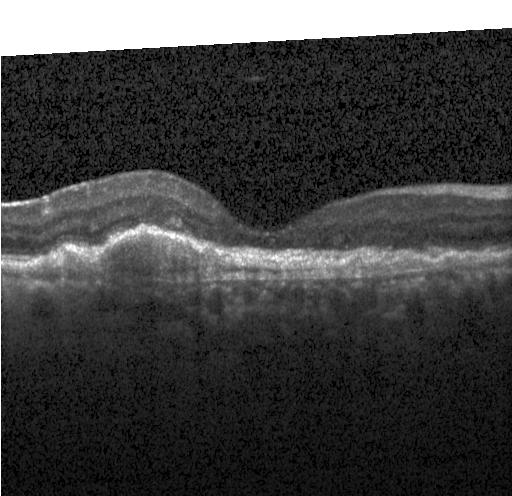
Heidelberg Spectralis · OCT B-scan · SD-OCT.
Finding: a choroidal neovascular membrane.